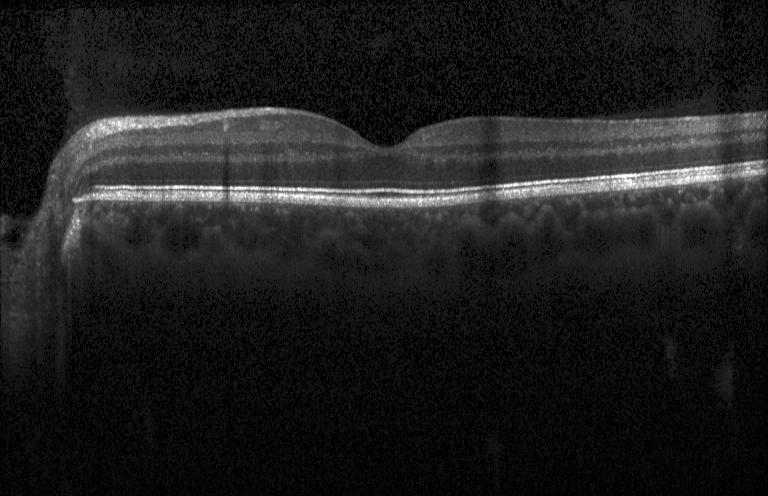

Heidelberg Spectralis. Optical coherence tomography scan. Spectral-domain OCT. Finding: no evidence of CNV, DME, or drusen.